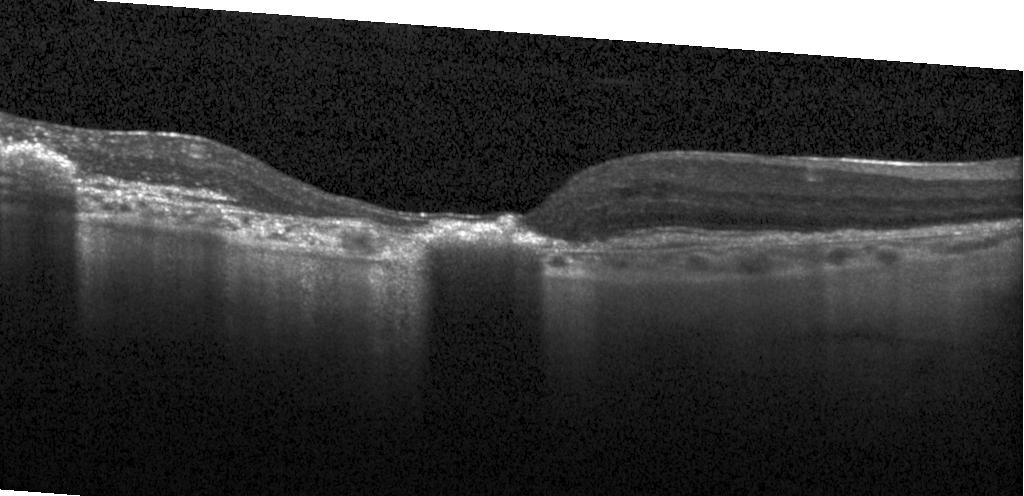 Impression: CNV.